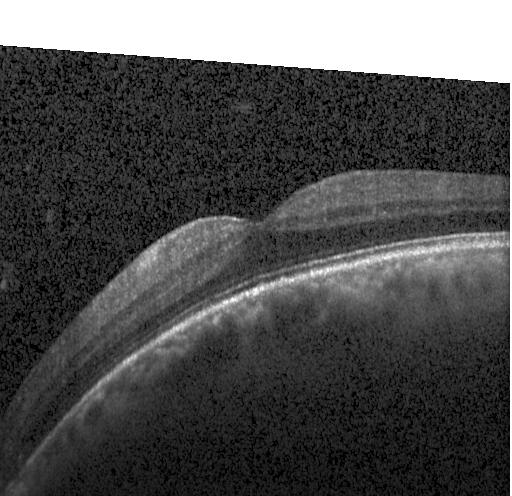 Heidelberg Spectralis OCT system · retinal OCT B-scan.
Diagnosis: no evidence of CNV, DME, or drusen.